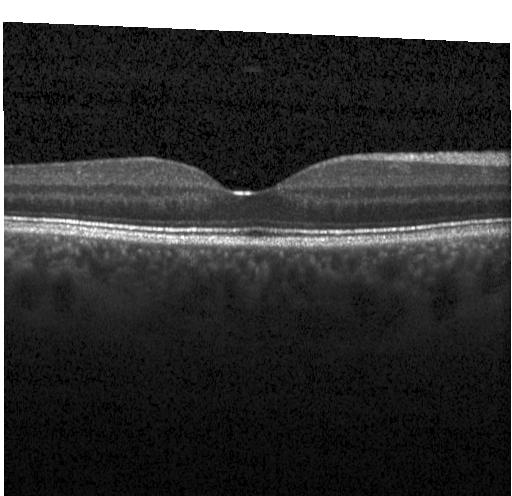

Optical coherence tomography B-scan · macular scan — Finding: no evidence of choroidal neovascularization, diabetic macular edema, or drusen.